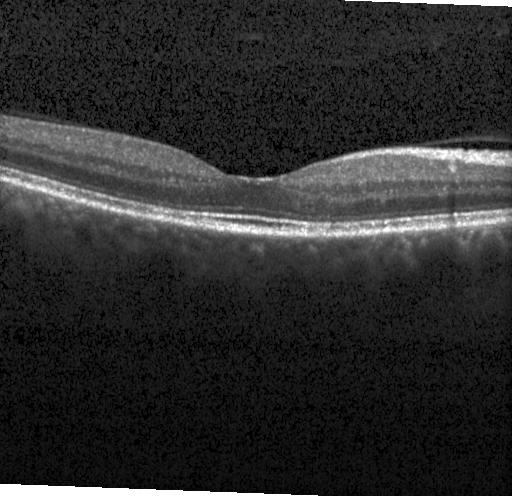 Spectral-domain optical coherence tomography; through the macula; retinal OCT cross-section; Heidelberg Spectralis.
Finding: no CNV, no DME, and no drusen.